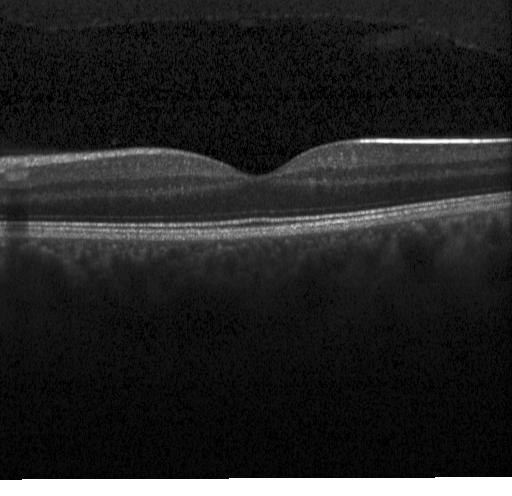

Dx: no evidence of choroidal neovascularization, diabetic macular edema, or drusen.